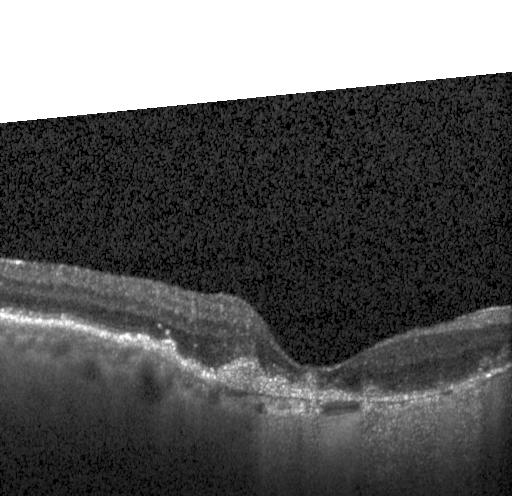 Retinal OCT B-scan
Dx: a choroidal neovascular membrane.